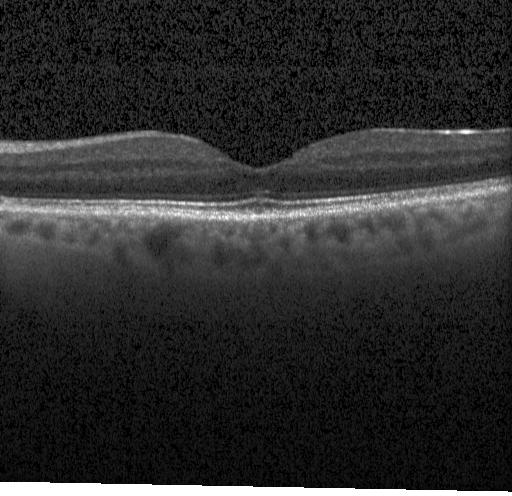 Retinal OCT cross-section
Macular OCT: no evidence of CNV, DME, or drusen.